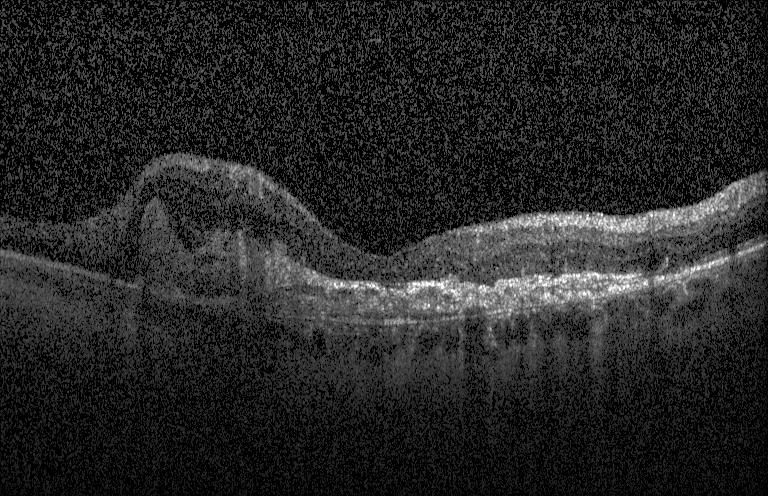 OCT finding: choroidal neovascularization.